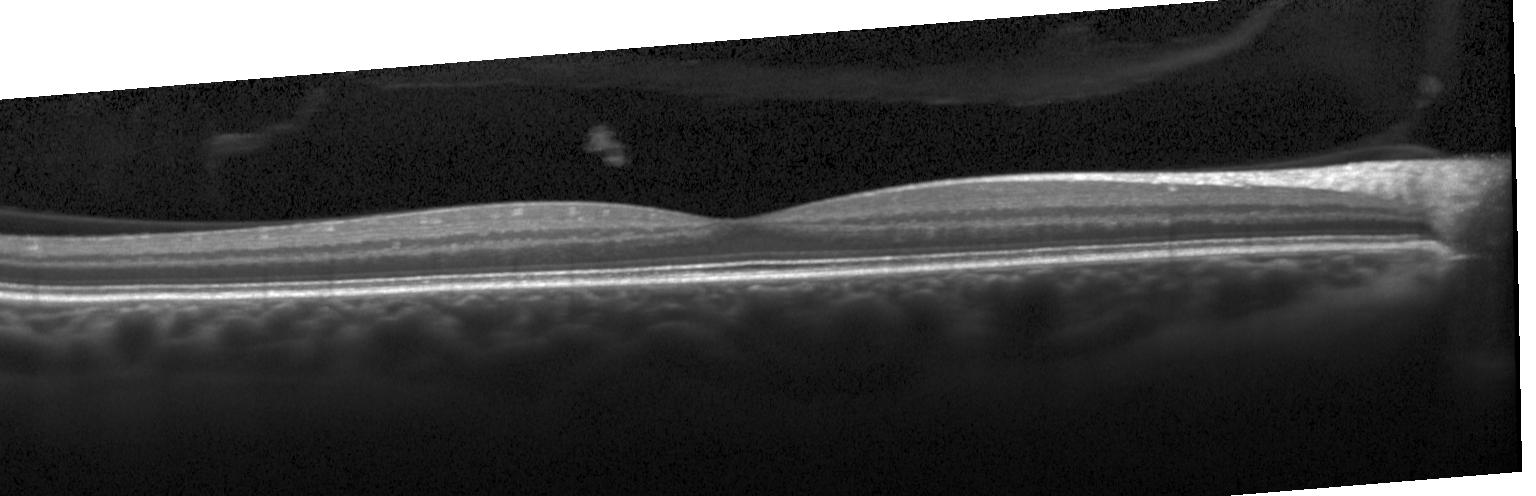 Spectral-domain OCT · instrument: Heidelberg Spectralis · optical coherence tomography scan · macular scan — Finding: no choroidal neovascularization, no diabetic macular edema, and no drusen.